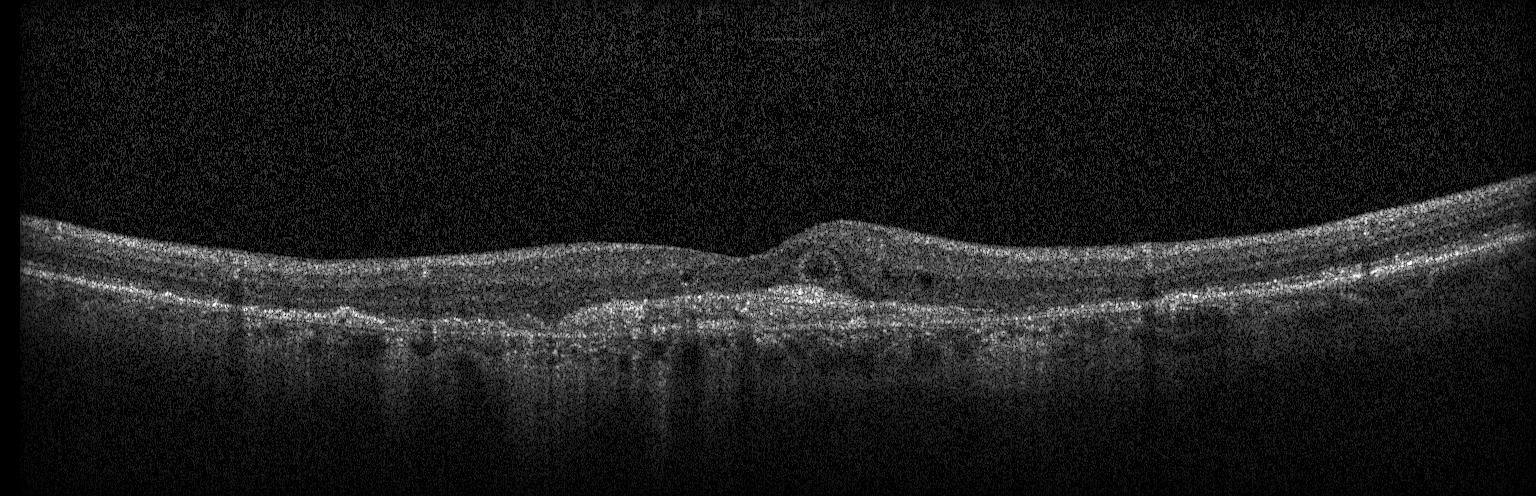

Optical coherence tomography scan. Fovea-centered. Instrument: Heidelberg Spectralis.
Dx: CNV.